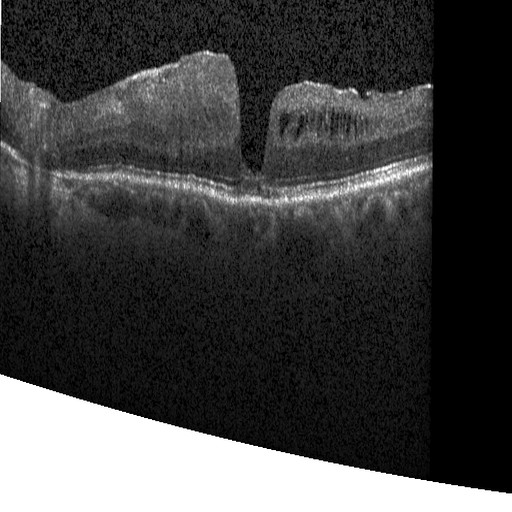
OCT line scan, acquired on a Heidelberg Spectralis, horizontal scan through the fovea, spectral-domain optical coherence tomography.
Diagnosis: diabetic macular edema.